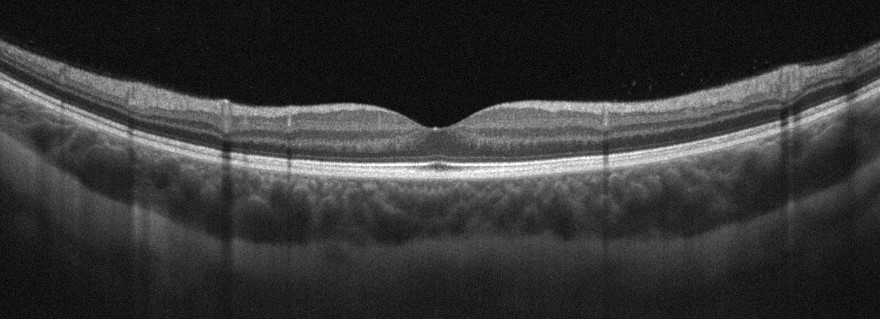

Instrument: Optovue Avanti RTVue XR; fovea-centered; retinal OCT B-scan.
Absence of AMD, DME, ERM, RAO, RVO, and vitreomacular interface disease.